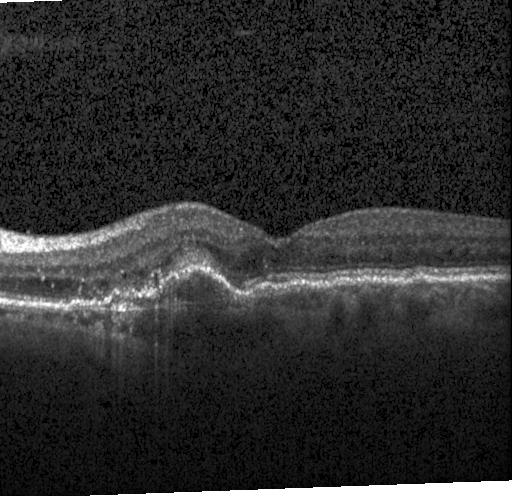

Heidelberg Spectralis OCT system. Retinal OCT cross-section
Diagnosis: CNV.